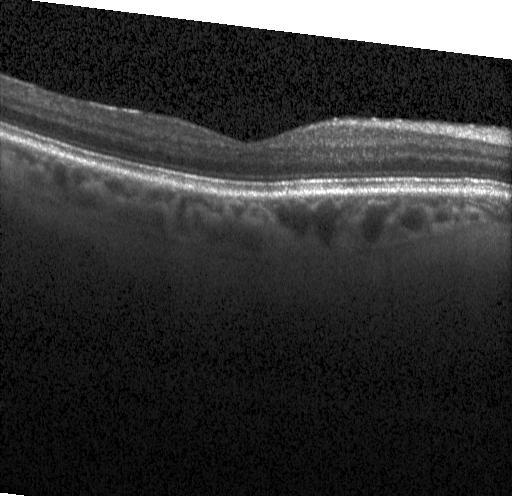
OCT B-scan. Finding: neither CNV, DME, nor drusen.